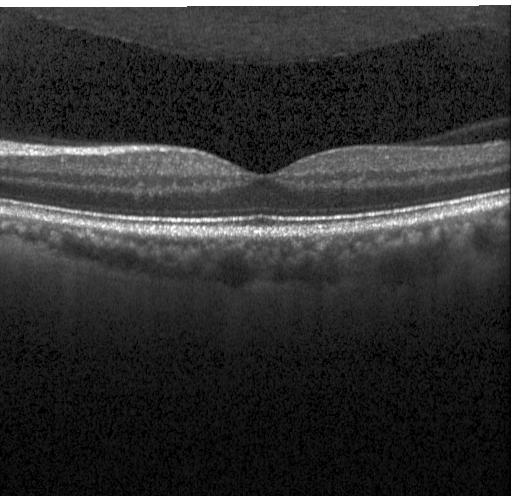
OCT line scan. Neither choroidal neovascularization, diabetic macular edema, nor drusen.